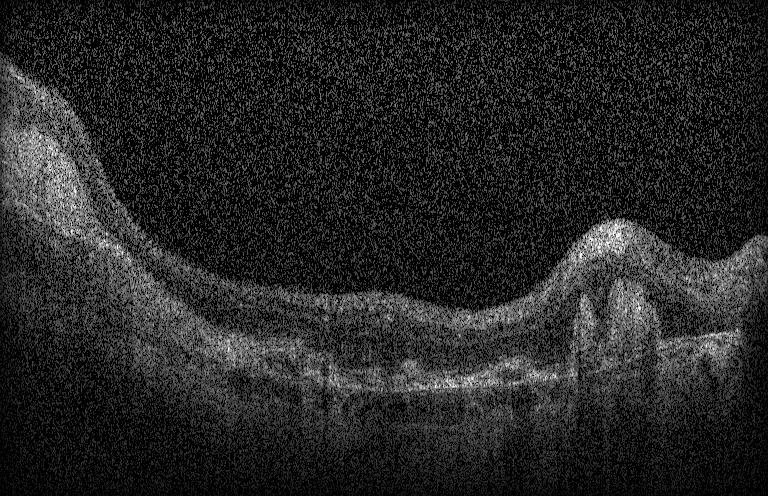

Finding: choroidal neovascularization (CNV).